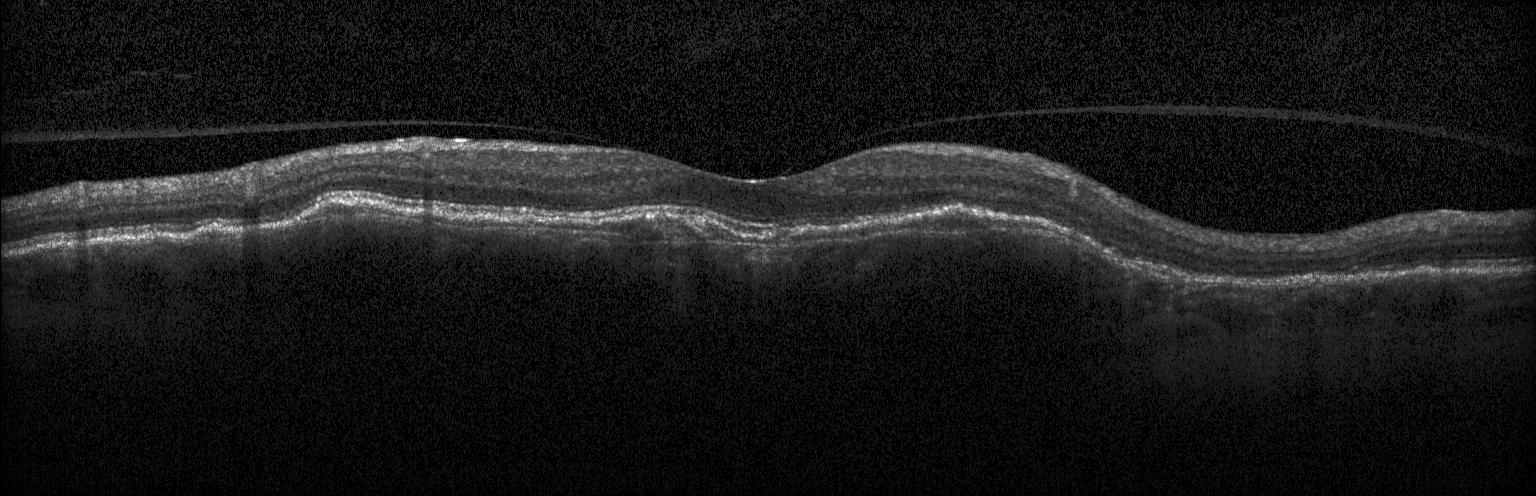
Spectral-domain OCT B-scan: choroidal neovascularization.